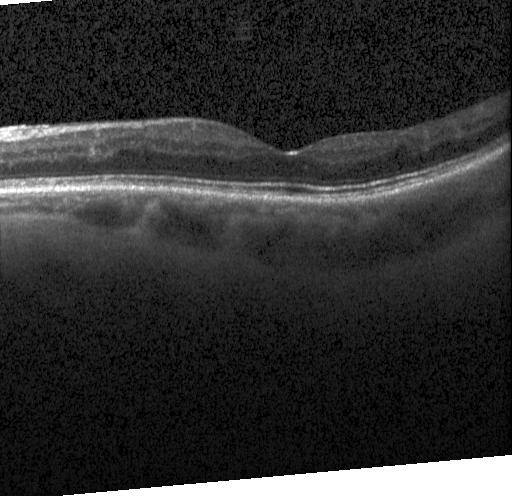
Impression: no evidence of choroidal neovascularization, diabetic macular edema, or drusen.